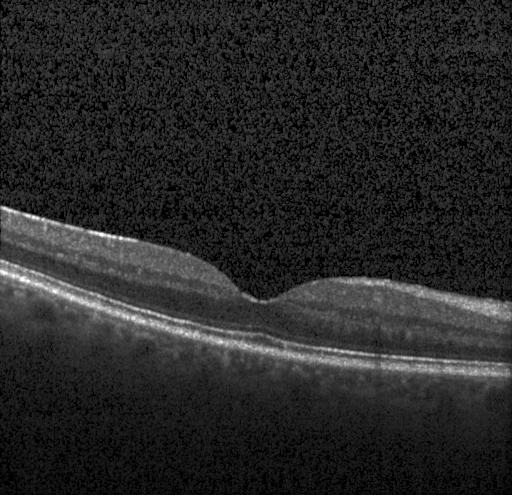 Retinal OCT cross-section. Finding: neither choroidal neovascularization, diabetic macular edema, nor drusen.